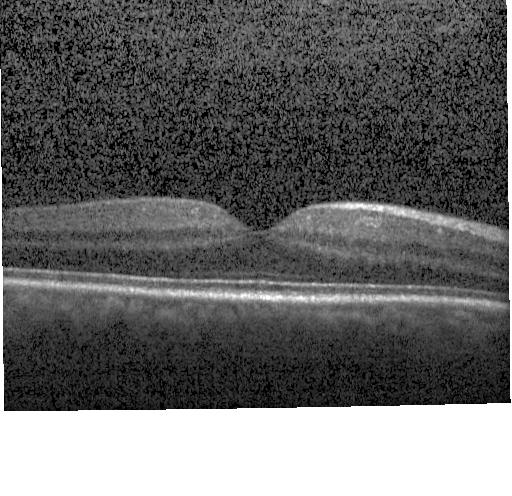
Impression: no choroidal neovascularization, no diabetic macular edema, and no drusen.